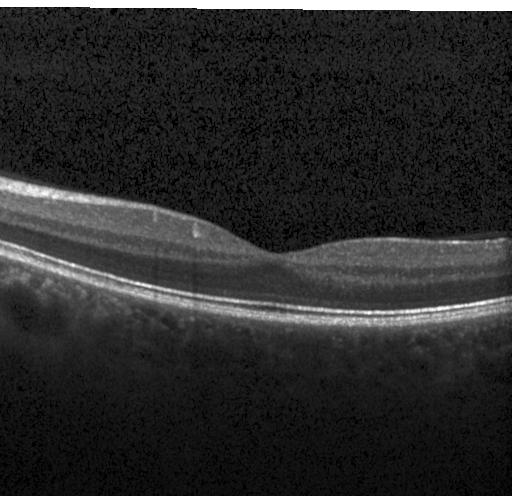
OCT line scan.
Diagnosis: no choroidal neovascularization, diabetic macular edema, or drusen.